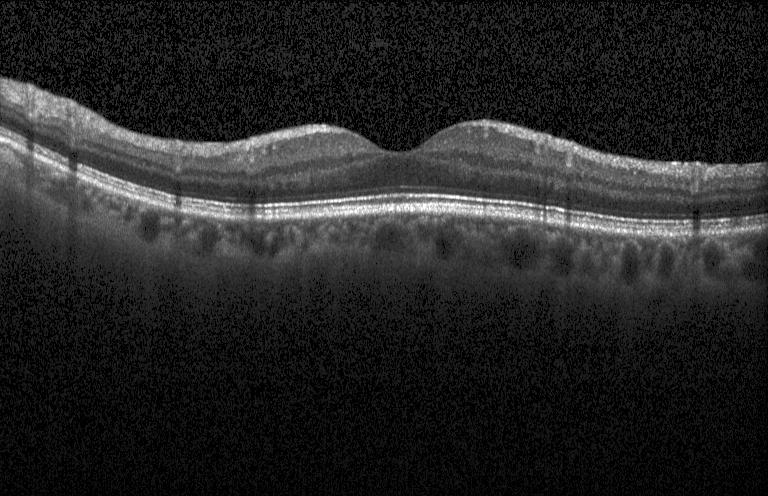
OCT line scan; spectral-domain optical coherence tomography.
Finding: neither choroidal neovascularization, diabetic macular edema, nor drusen.